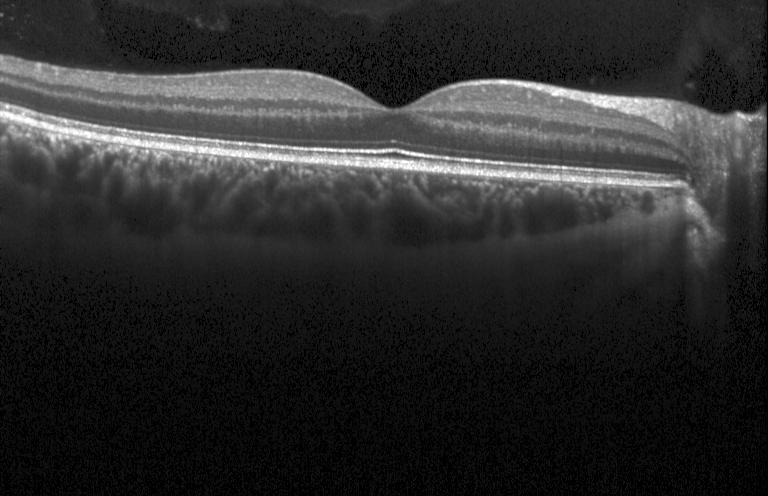 Macular OCT: no evidence of choroidal neovascularization, diabetic macular edema, or drusen.